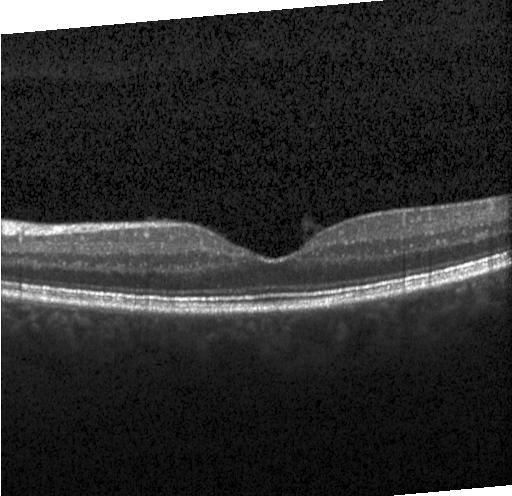

Horizontal scan through the fovea. Spectral-domain OCT. Heidelberg Spectralis. Optical coherence tomography scan — No evidence of choroidal neovascularization, diabetic macular edema, or drusen.